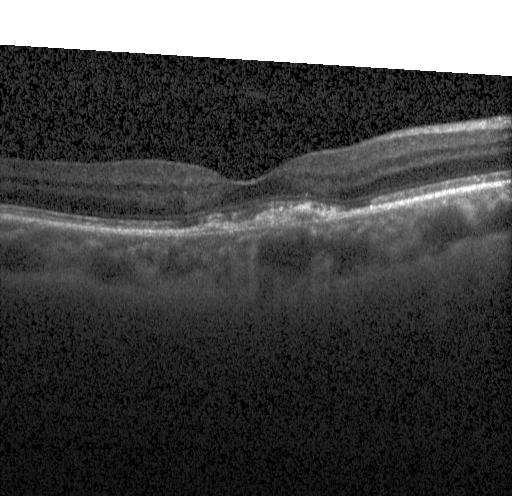

This B-scan demonstrates choroidal neovascularization (CNV).